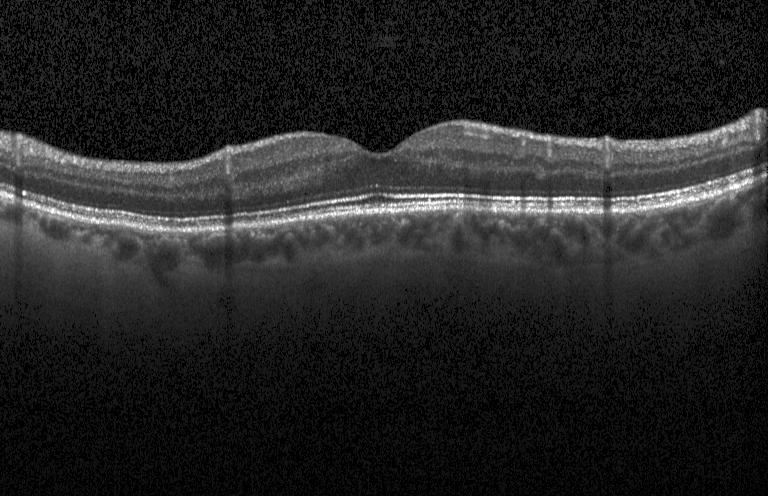
Retinal OCT cross-section. Diagnosis: no choroidal neovascularization, no diabetic macular edema, and no drusen.